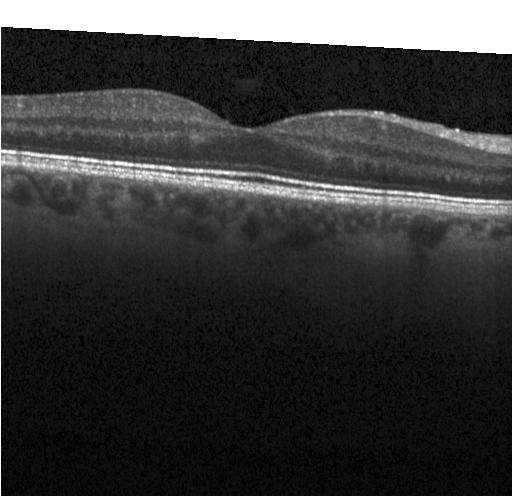

Spectral-domain OCT B-scan: neither choroidal neovascularization, diabetic macular edema, nor drusen.